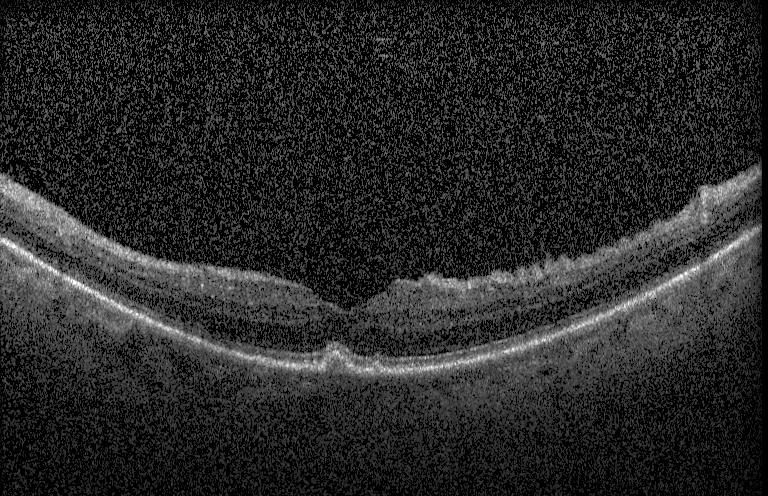
Dx: drusen.